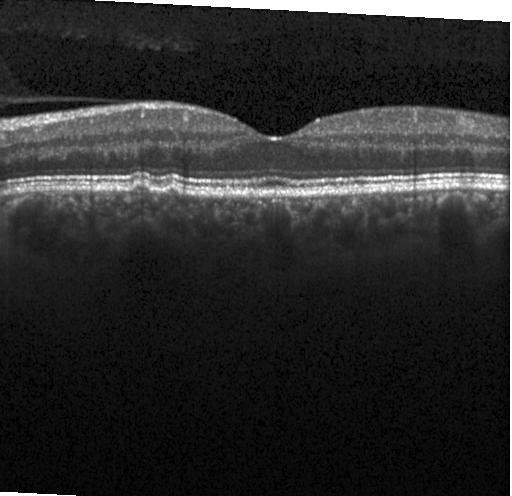
OCT line scan
Finding: drusen.